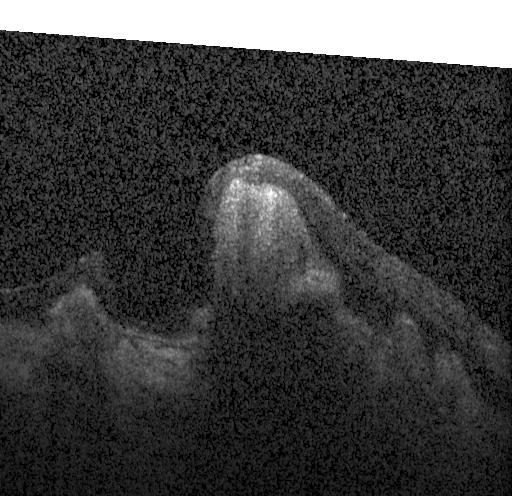
Diagnosis: choroidal neovascularization.